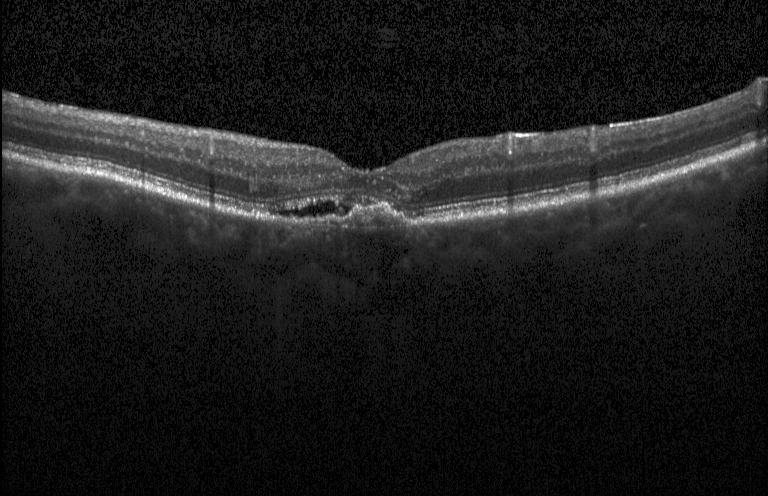 Through the macula; instrument: Heidelberg Spectralis; spectral-domain optical coherence tomography; optical coherence tomography scan
Diagnosis: CNV.